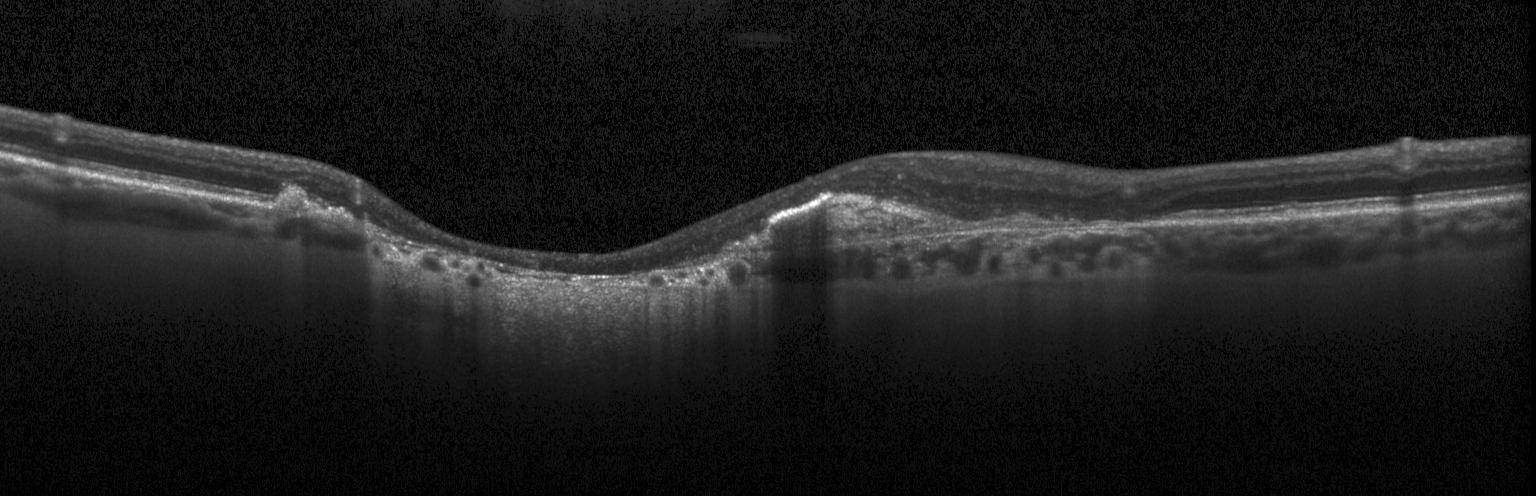 OCT B-scan showing choroidal neovascularization (CNV).